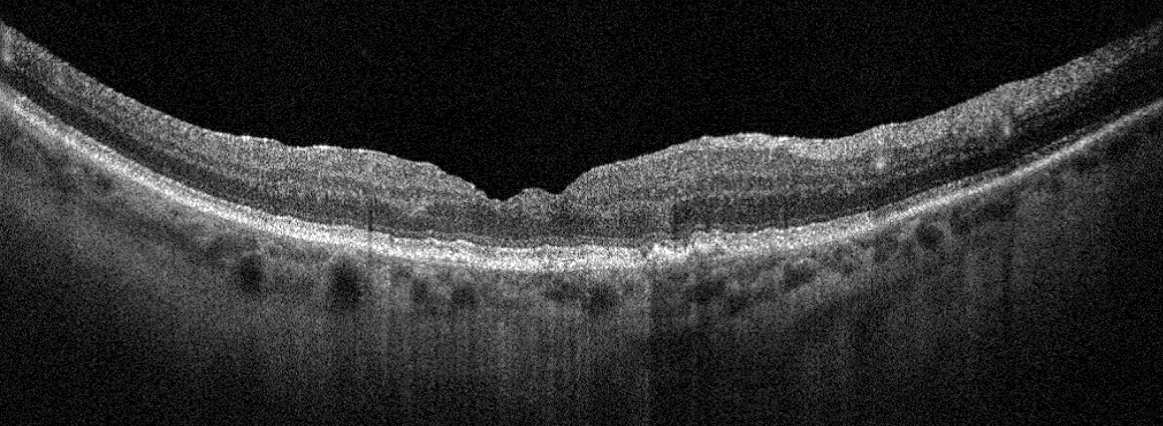 Retinal OCT cross-section. Oculus dexter — Age-related macular degeneration.